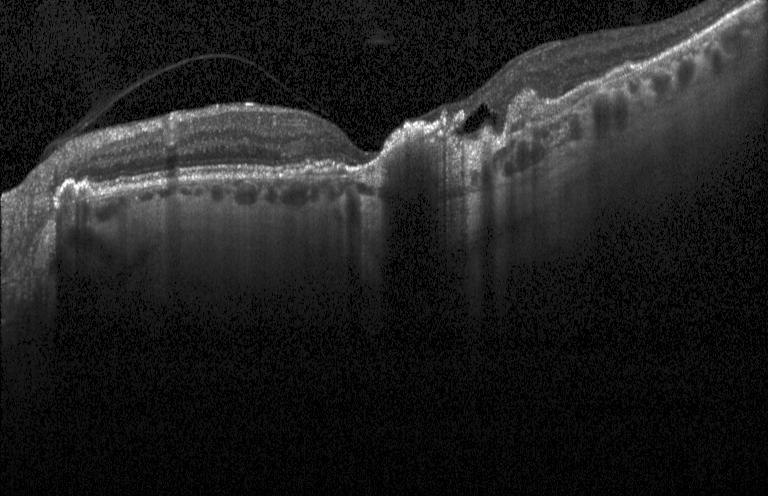 Choroidal neovascularization (CNV).